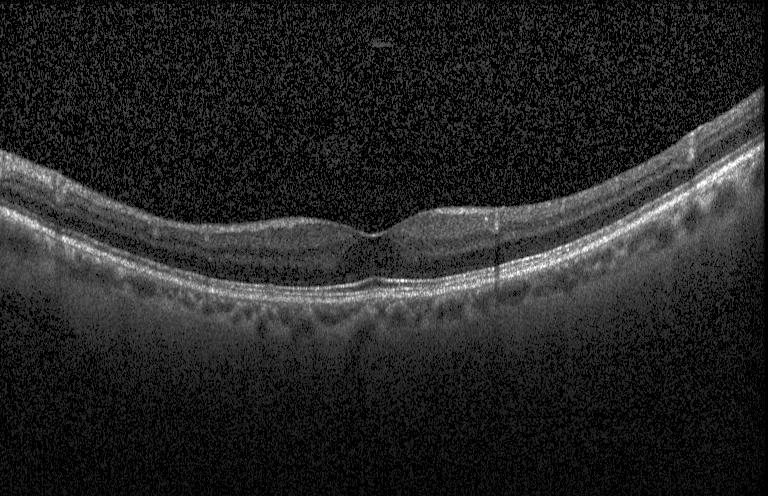
OCT finding: no evidence of CNV, DME, or drusen.